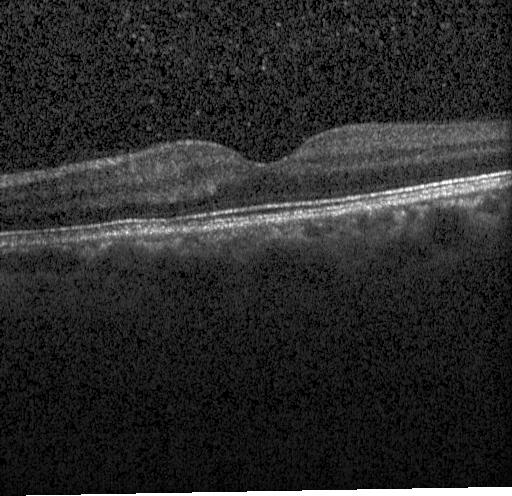 Heidelberg Spectralis OCT system. OCT B-scan. Spectral-domain optical coherence tomography. Macular scan
Impression: no choroidal neovascularization, diabetic macular edema, or drusen.